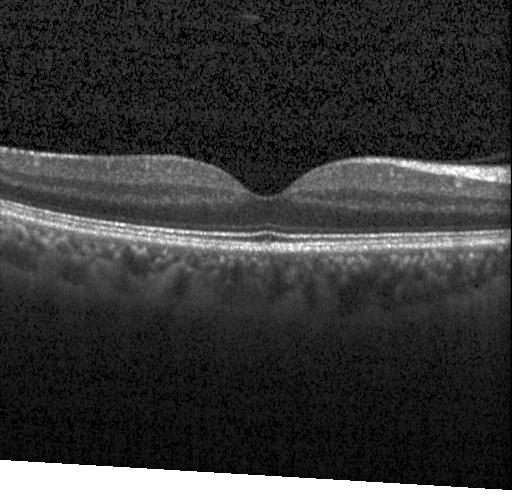 Retinal OCT B-scan · SD-OCT · instrument: Heidelberg Spectralis · fovea-centered
Diagnosis: no choroidal neovascularization, diabetic macular edema, or drusen.